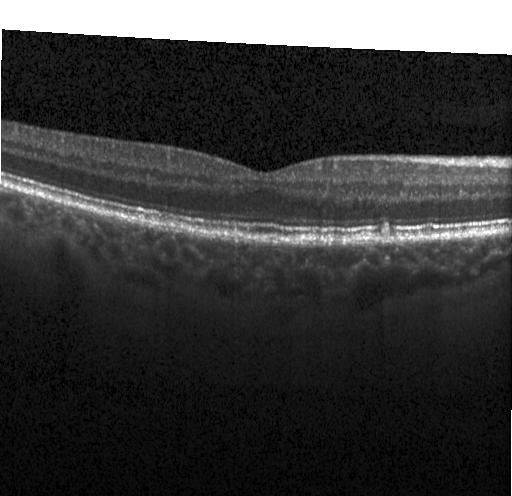

Macular OCT demonstrating drusen.